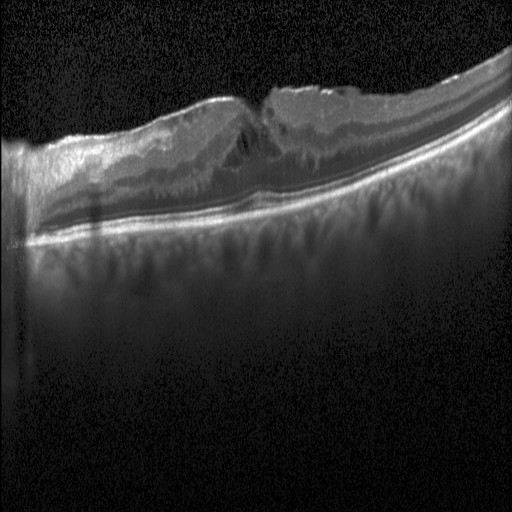 OCT line scan — Diagnosis: diabetic macular edema (DME).